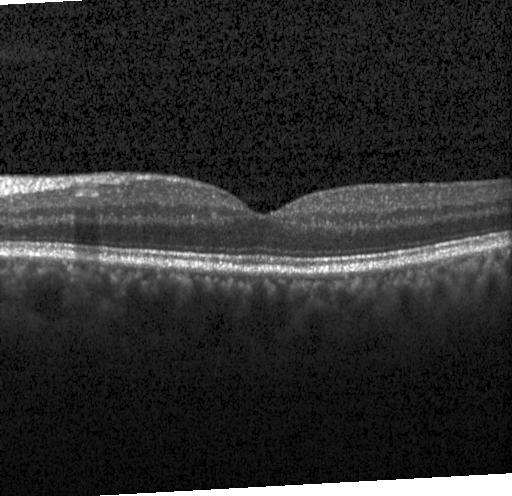

Retinal OCT B-scan · horizontal scan through the fovea · Heidelberg Spectralis — Neither choroidal neovascularization, diabetic macular edema, nor drusen.